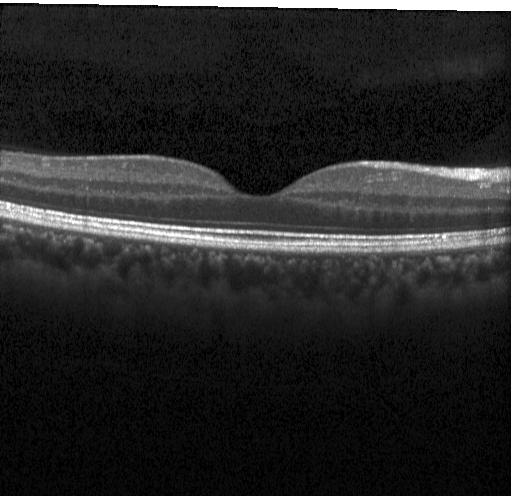

Horizontal scan through the fovea, spectral-domain optical coherence tomography, retinal OCT cross-section, instrument: Heidelberg Spectralis.
Impression: neither choroidal neovascularization, diabetic macular edema, nor drusen.